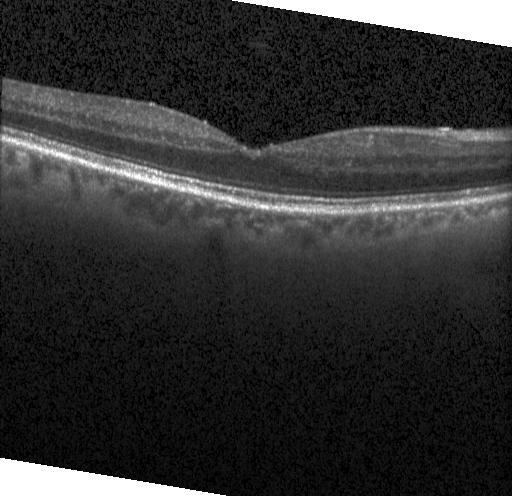 Retinal OCT cross-section. Finding: neither choroidal neovascularization, diabetic macular edema, nor drusen.